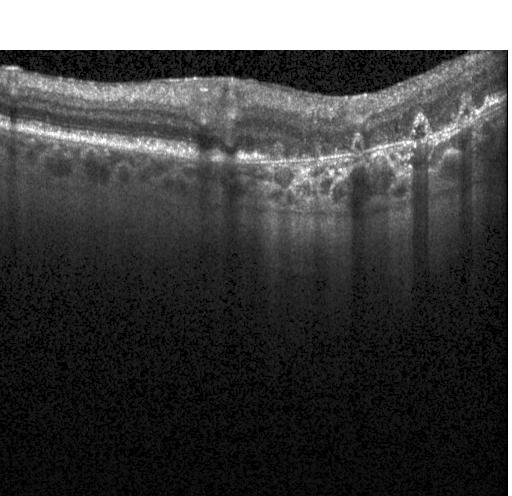 Dx: a choroidal neovascular membrane.